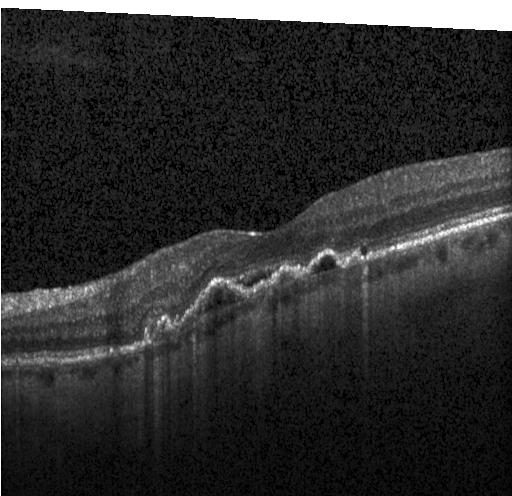
Assessment: a choroidal neovascular membrane.